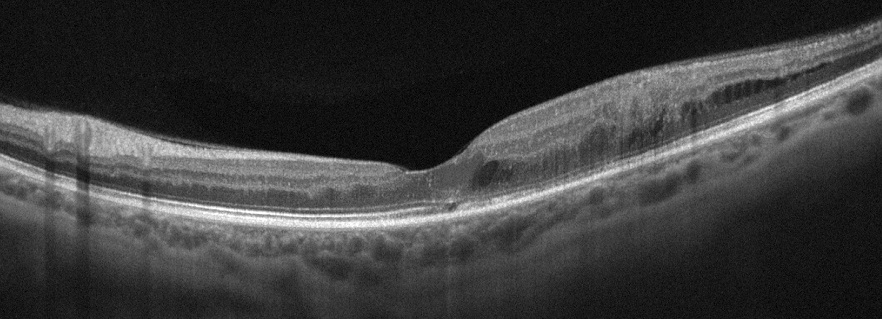
Optical coherence tomography scan. Optovue Avanti RTVue XR. Fovea-centered.
Diagnosis: diabetic macular edema (DME).